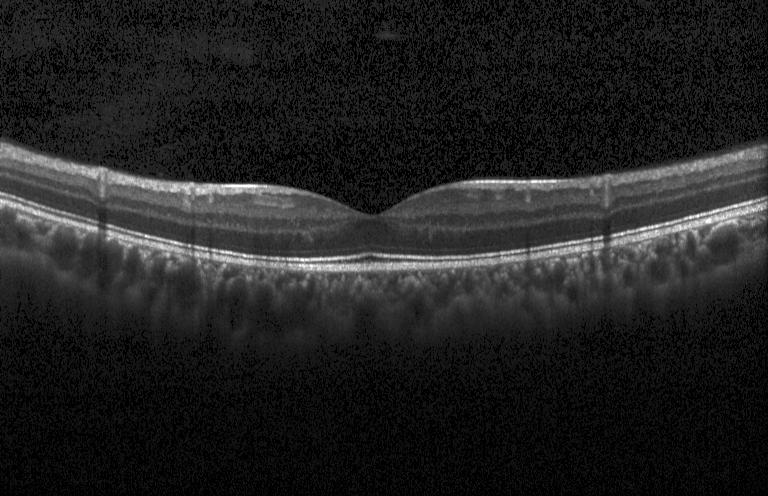
Macular OCT: no CNV, DME, or drusen.